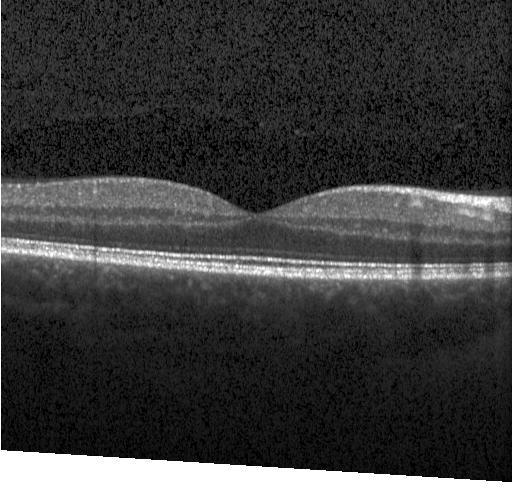

Macular OCT: no CNV, no DME, and no drusen.